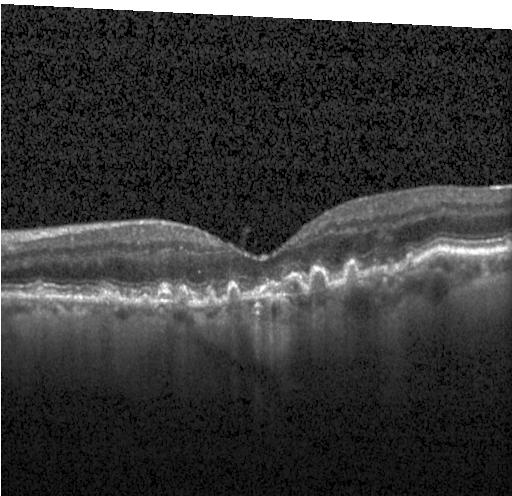 Retinal OCT B-scan. This B-scan demonstrates sub-RPE drusenoid deposits.